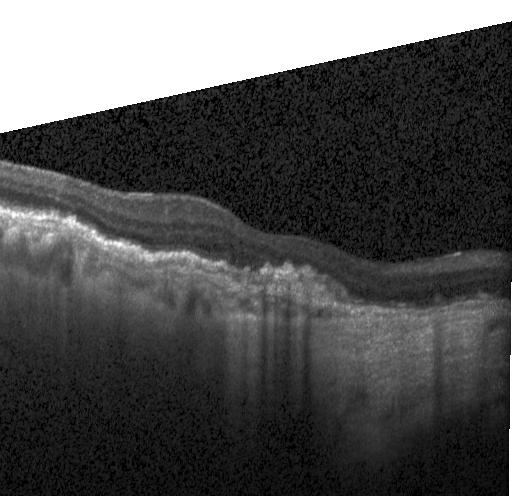 Spectral-domain OCT, OCT B-scan
The scan shows a choroidal neovascular membrane.